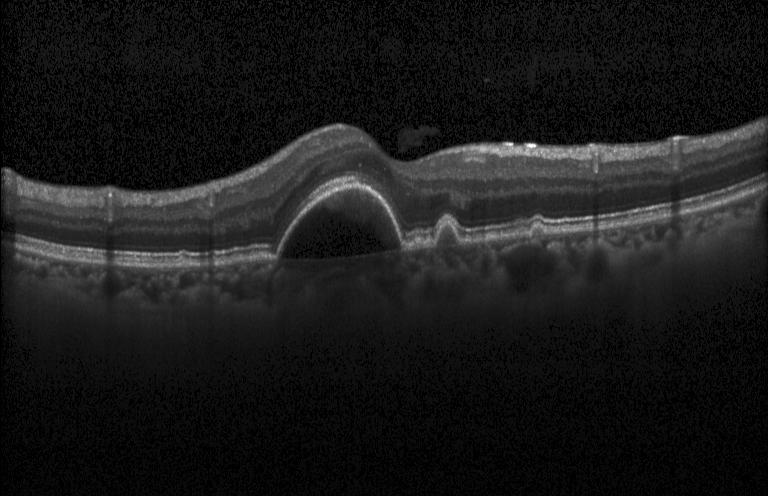
OCT finding: a choroidal neovascular membrane.